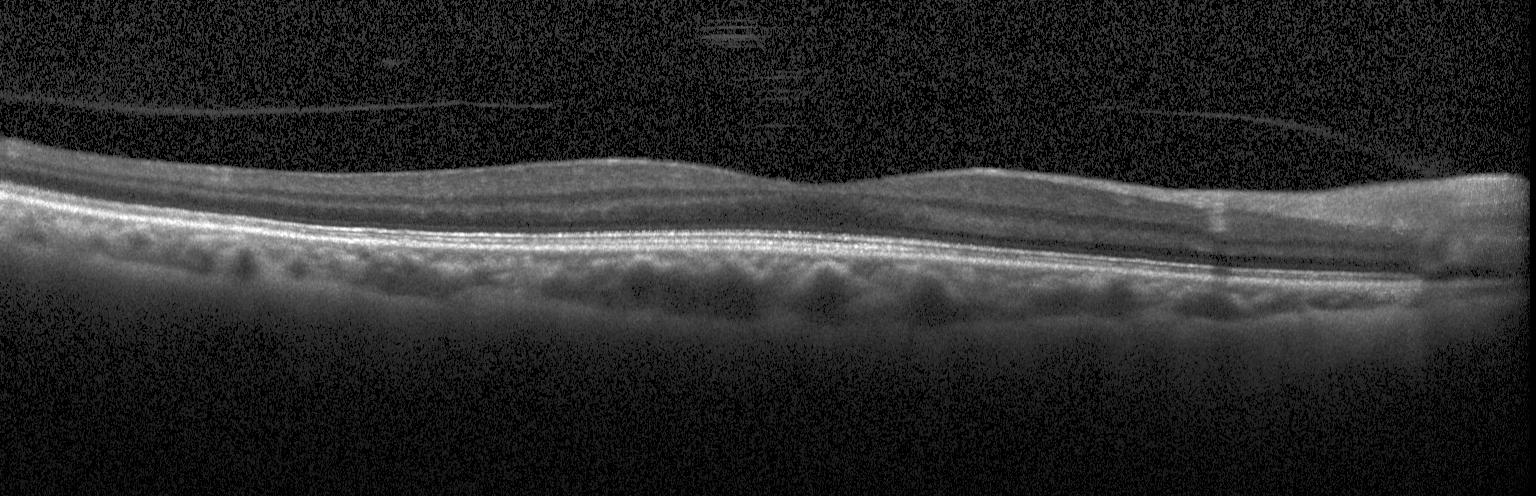
Spectral-domain OCT. Retinal OCT B-scan. Centered on the fovea. Heidelberg Spectralis
Finding: no CNV, no DME, and no drusen.